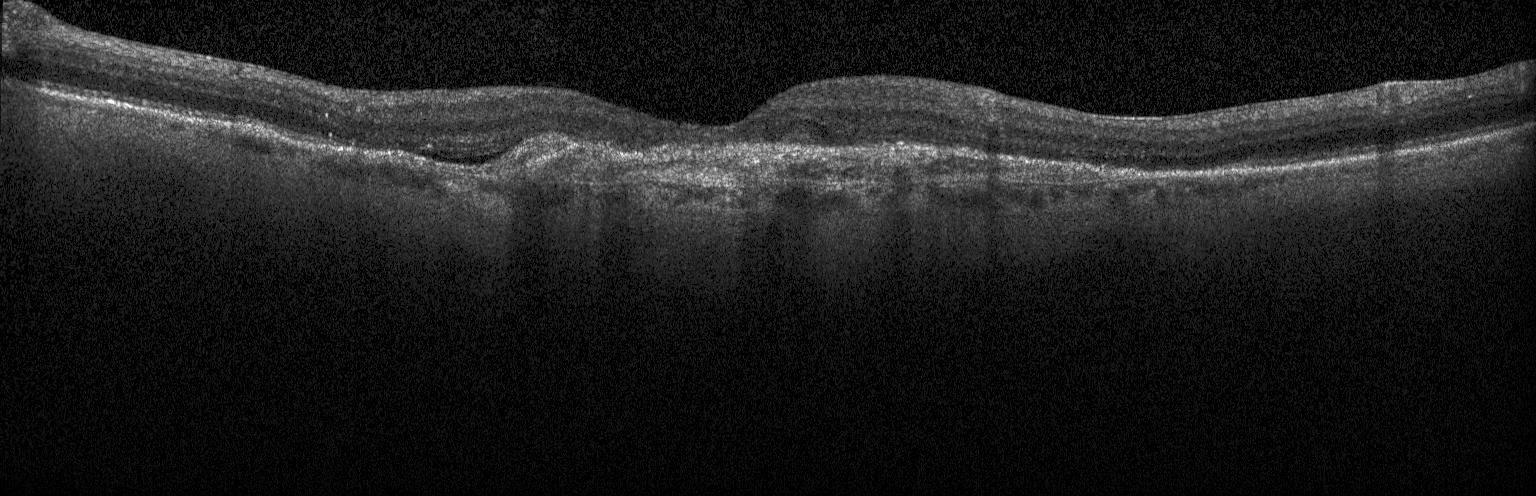

Finding: a choroidal neovascular membrane.